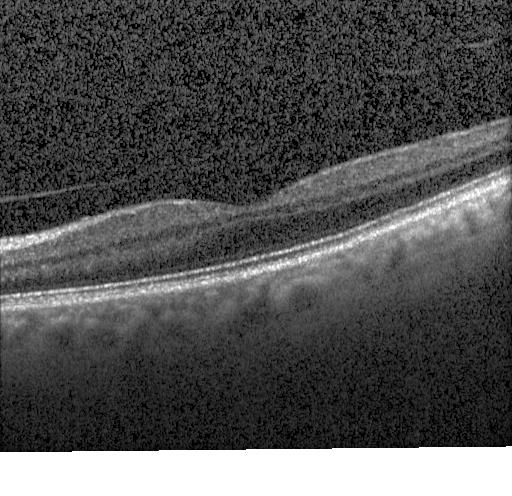
OCT B-scan · macular scan. OCT finding: no evidence of CNV, DME, or drusen.